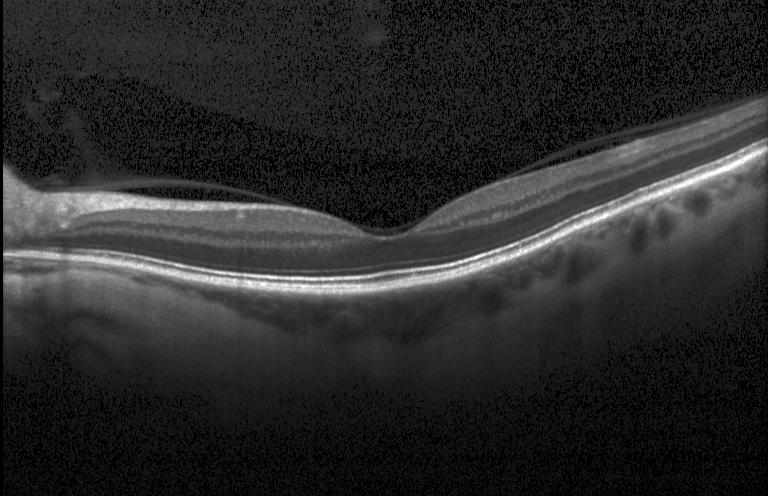
Spectral-domain OCT, optical coherence tomography B-scan, fovea-centered, Heidelberg Spectralis OCT system. Diagnosis: no evidence of choroidal neovascularization, diabetic macular edema, or drusen.